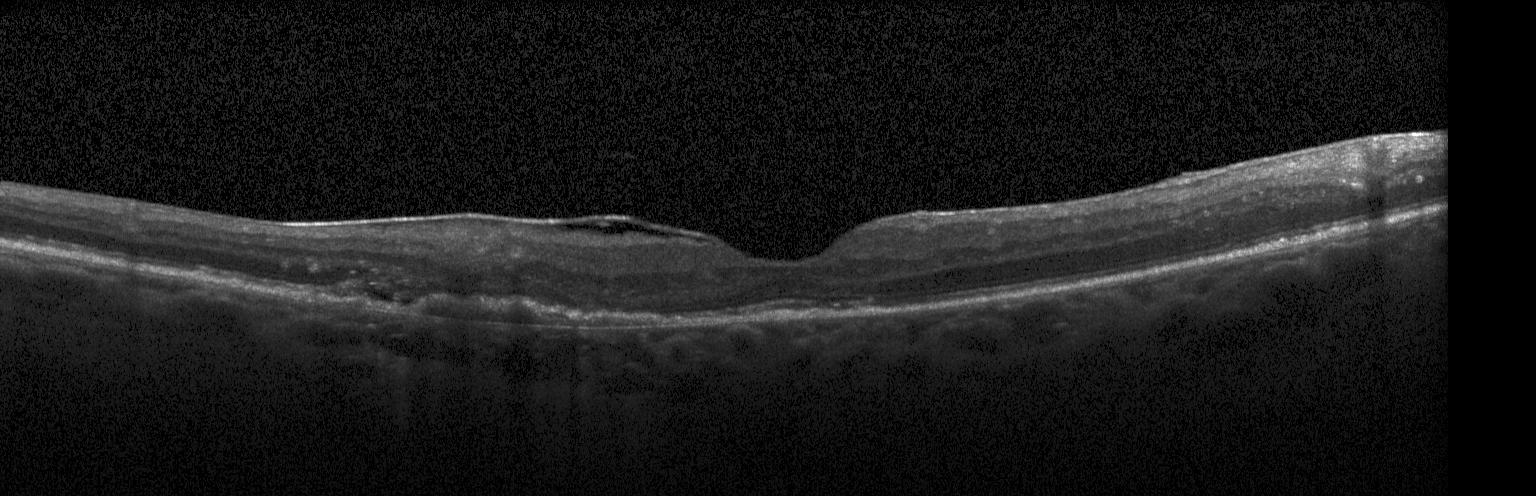 Impression: a choroidal neovascular membrane.